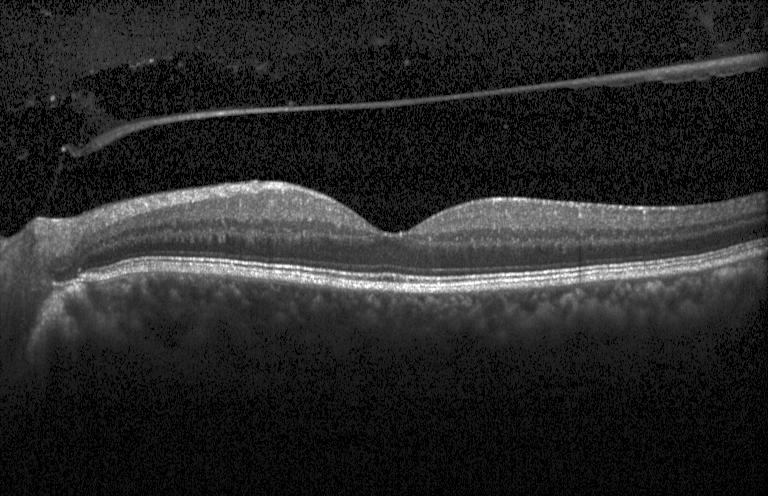 OCT B-scan · Heidelberg Spectralis OCT system
Dx: no evidence of choroidal neovascularization, diabetic macular edema, or drusen.